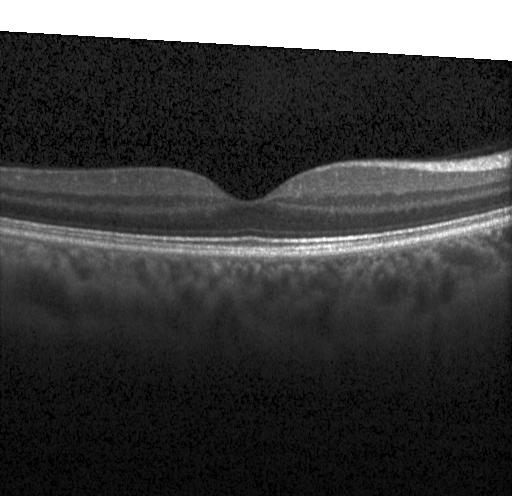
SD-OCT, acquired on a Heidelberg Spectralis, optical coherence tomography B-scan
Assessment: no CNV, no DME, and no drusen.